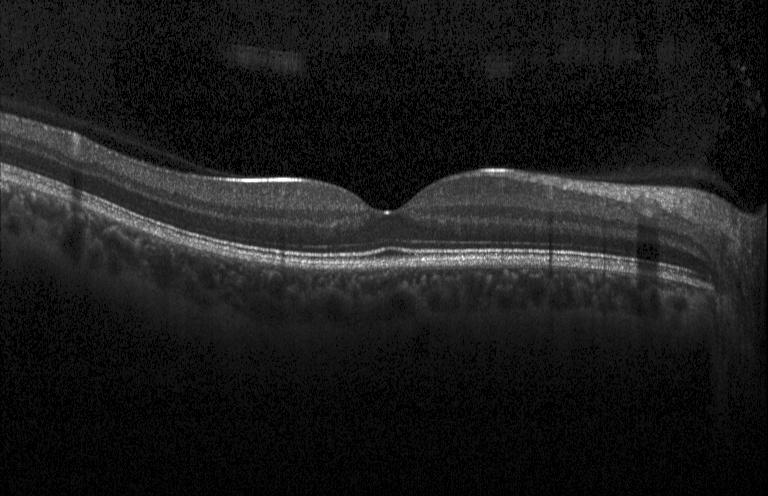
Heidelberg Spectralis OCT system, horizontal scan through the fovea, optical coherence tomography scan, SD-OCT. Finding: no choroidal neovascularization, no diabetic macular edema, and no drusen.